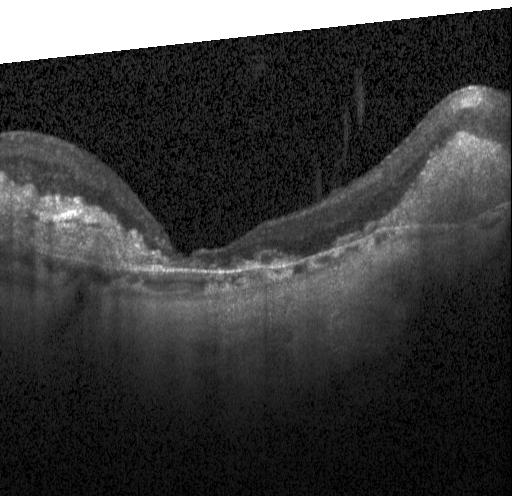

Spectral-domain OCT B-scan: a choroidal neovascular membrane.